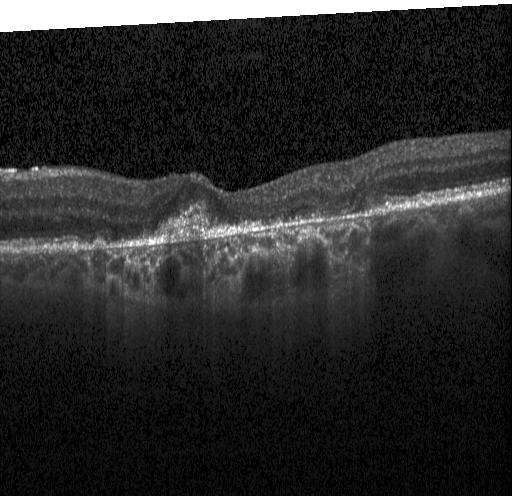 Finding: choroidal neovascularization.